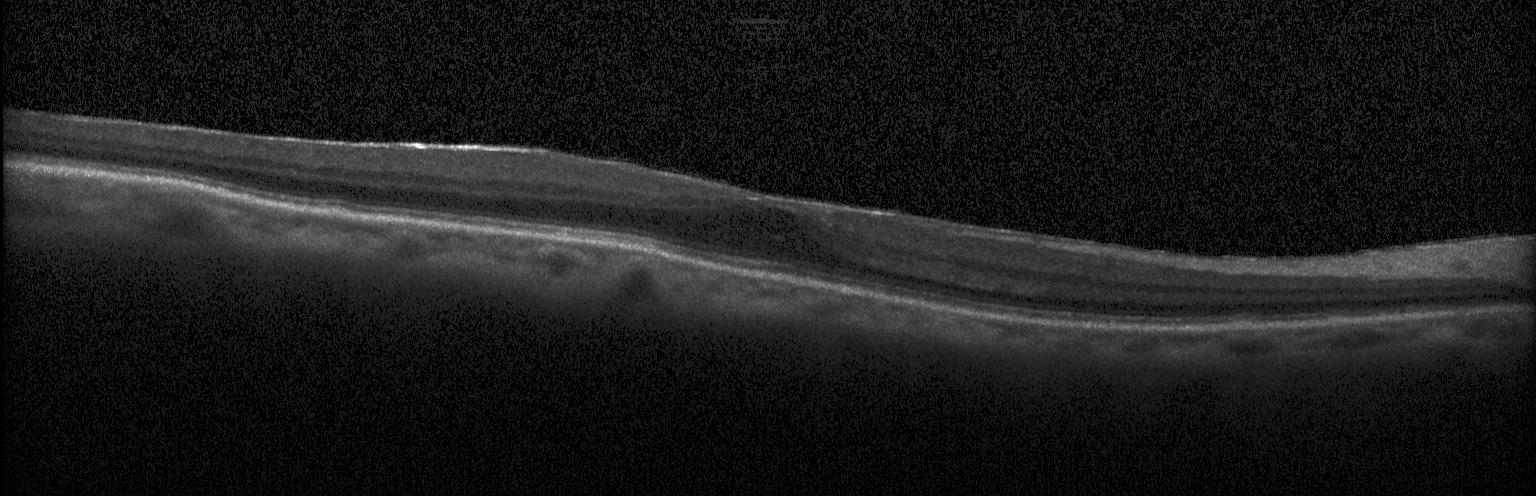

Macular OCT: diabetic macular edema (DME).